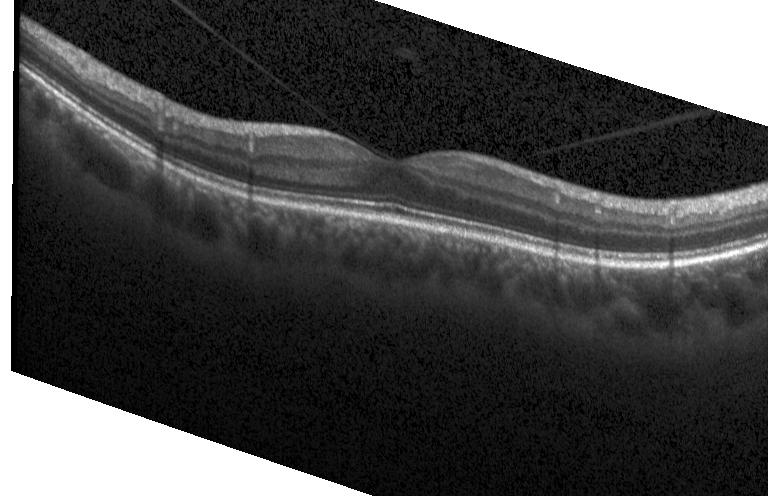

SD-OCT; Heidelberg Spectralis; OCT B-scan; centered on the fovea.
Impression: no CNV, no DME, and no drusen.